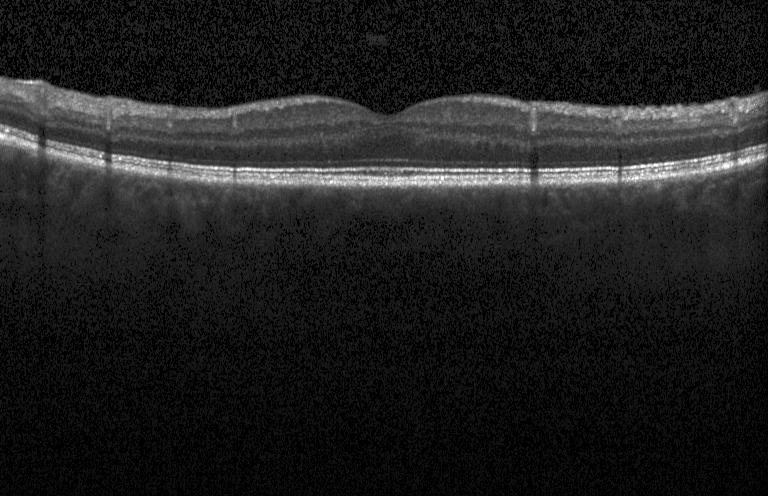 OCT scan showing no evidence of choroidal neovascularization, diabetic macular edema, or drusen.